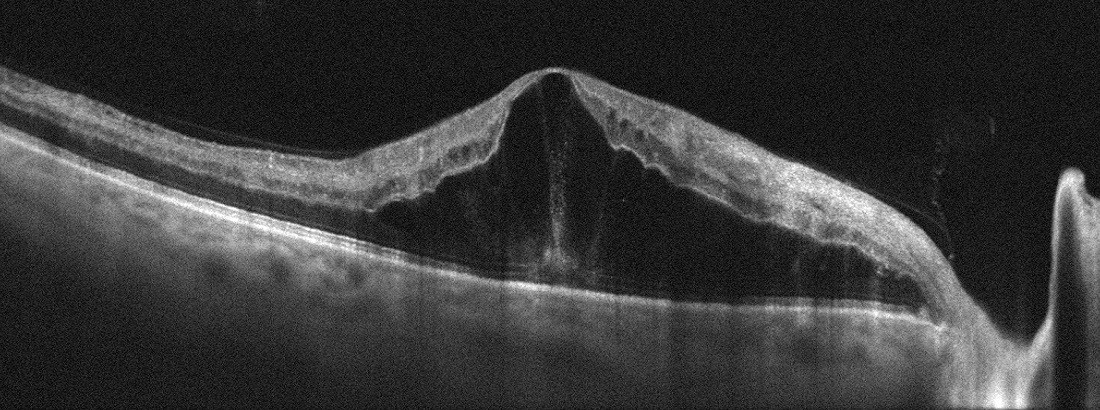 Retinal OCT B-scan. Through the macula
Finding: RVO.